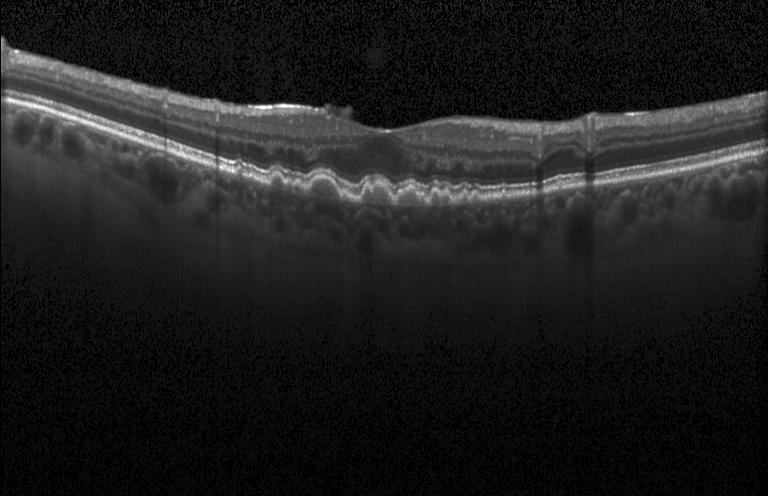
Spectral-domain optical coherence tomography · horizontal scan through the fovea · optical coherence tomography B-scan.
Finding: drusen.